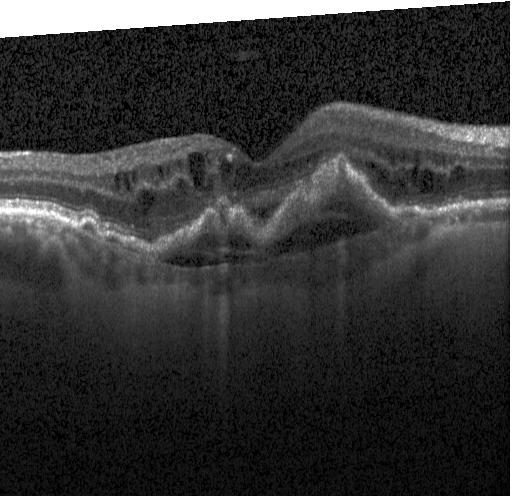

Optical coherence tomography scan, spectral-domain OCT. Impression: choroidal neovascularization.